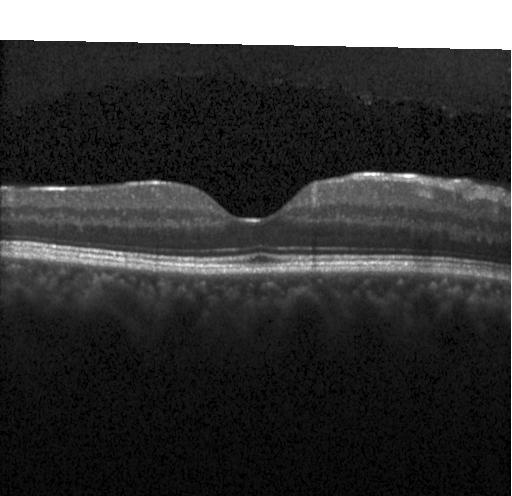
Instrument: Heidelberg Spectralis, spectral-domain OCT, retinal OCT B-scan — The scan shows no choroidal neovascularization, no diabetic macular edema, and no drusen.